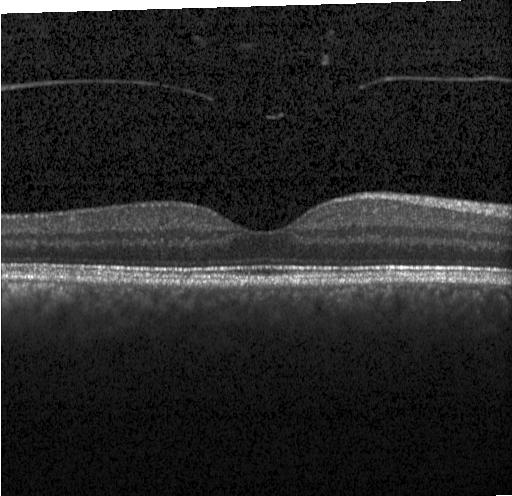 Diagnosis: neither choroidal neovascularization, diabetic macular edema, nor drusen.